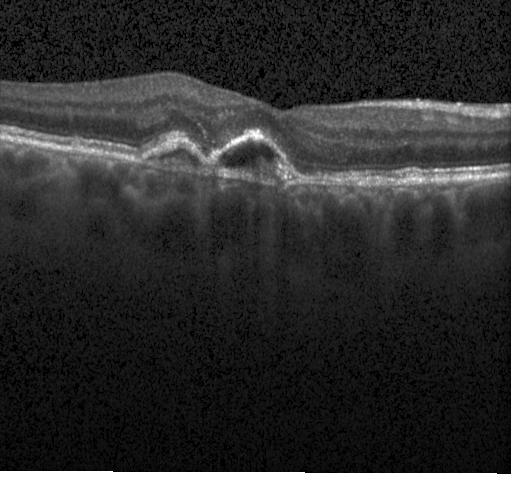

Heidelberg Spectralis OCT system; spectral-domain optical coherence tomography; optical coherence tomography B-scan; macular scan.
Impression: a choroidal neovascular membrane.